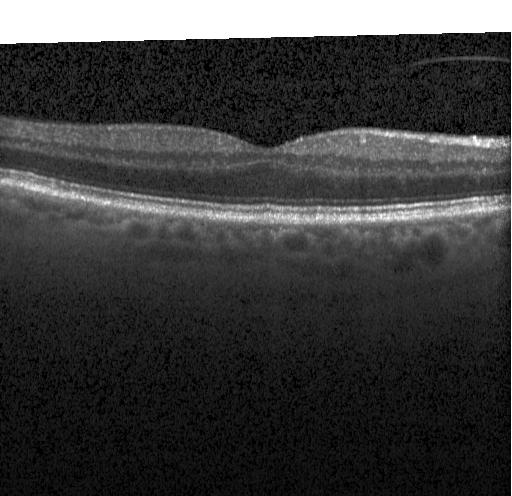

Retinal OCT cross-section showing no evidence of CNV, DME, or drusen.